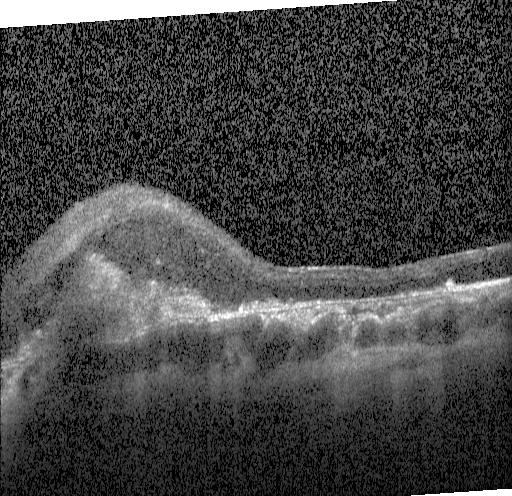
Macular OCT demonstrating choroidal neovascularization.